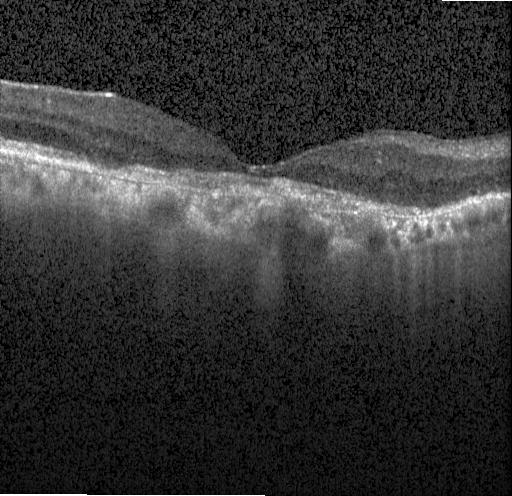
Spectral-domain OCT; acquired on a Heidelberg Spectralis; macular scan; optical coherence tomography scan
Macular OCT: choroidal neovascularization.